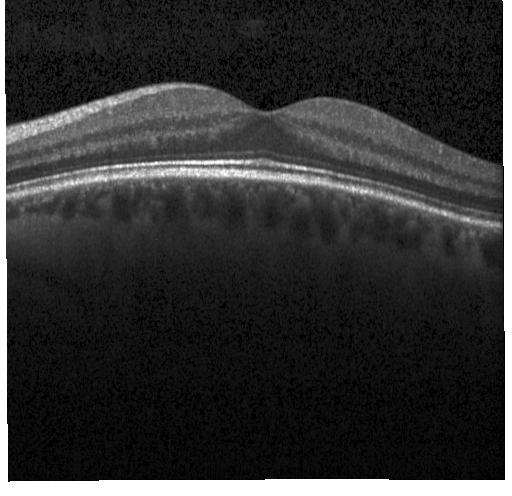

Dx: neither CNV, DME, nor drusen.